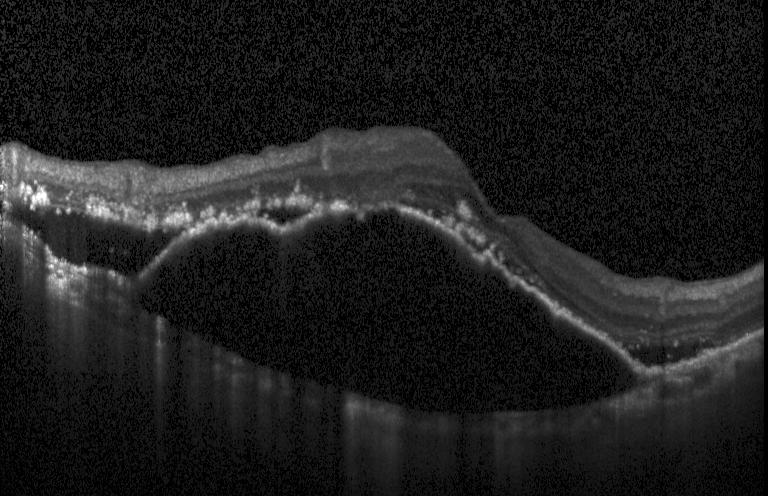 OCT line scan. Macular scan — Impression: CNV.